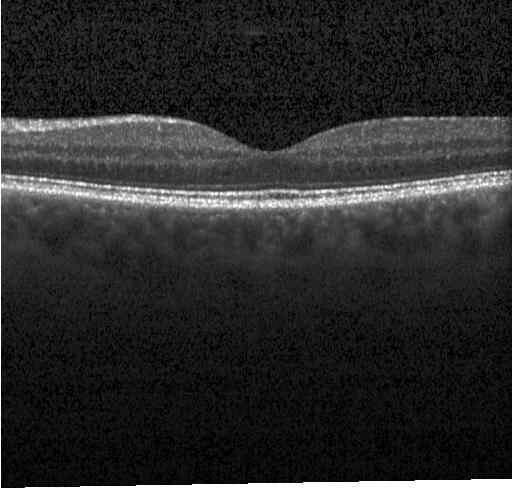 OCT B-scan; instrument: Heidelberg Spectralis. Impression: no CNV, DME, or drusen.